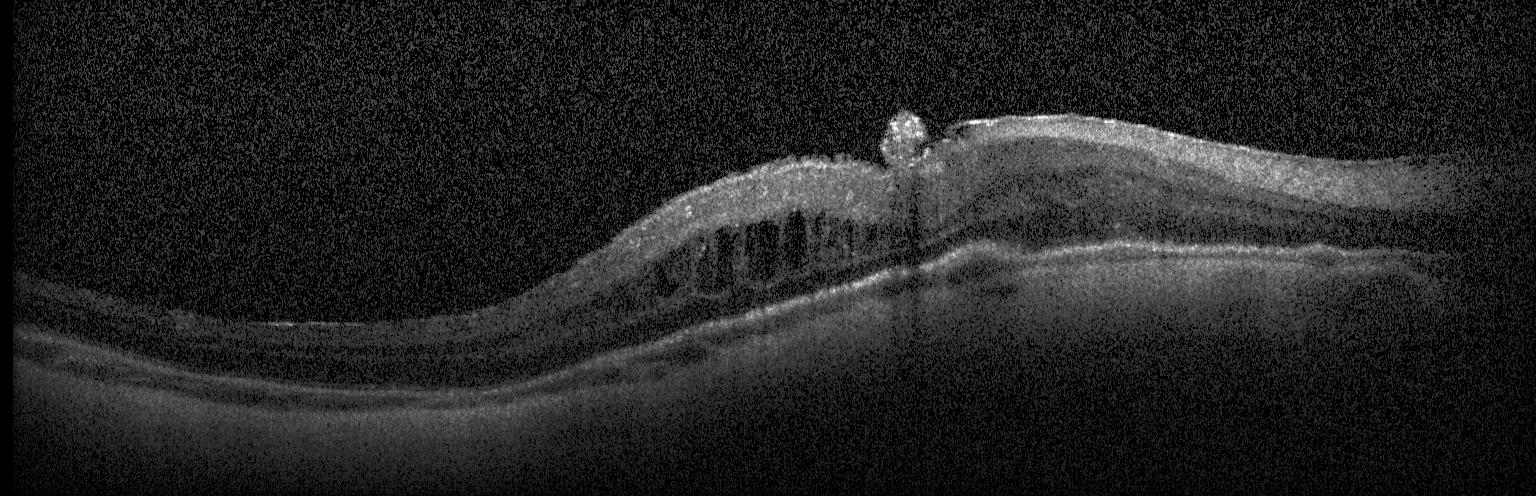

Dx: diabetic macular edema.